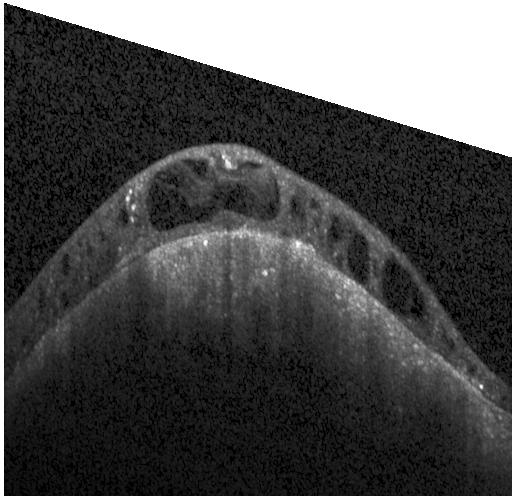 Optical coherence tomography B-scan, Heidelberg Spectralis, macular scan — Impression: diabetic macular edema.